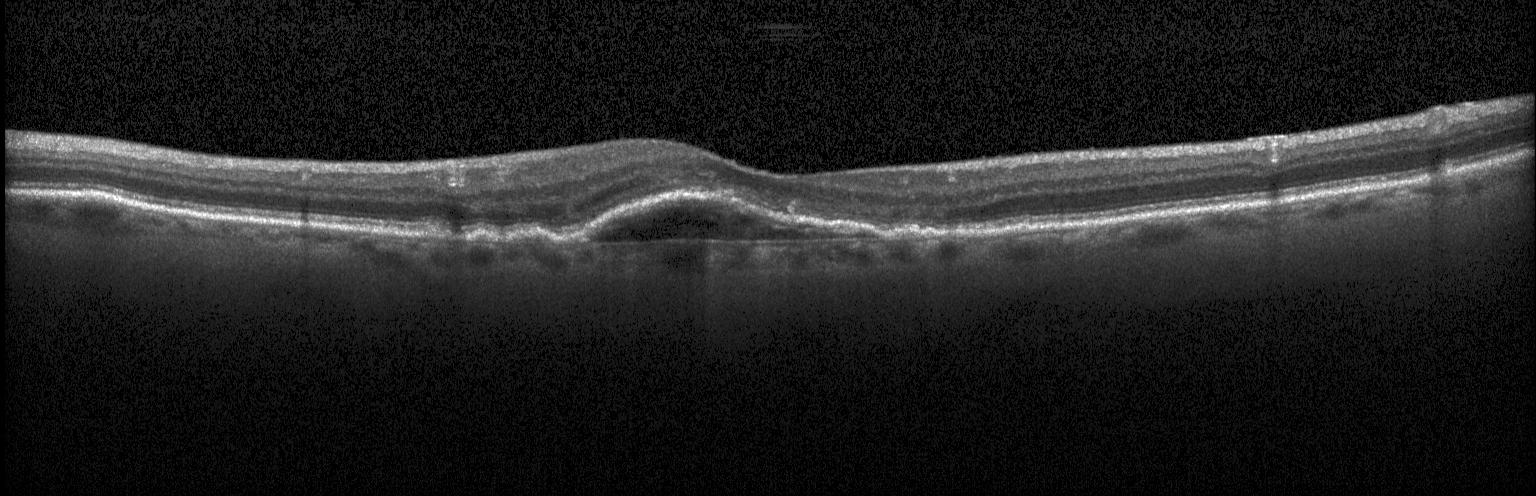 Spectral-domain OCT, instrument: Heidelberg Spectralis, optical coherence tomography scan, centered on the fovea. This B-scan demonstrates CNV.